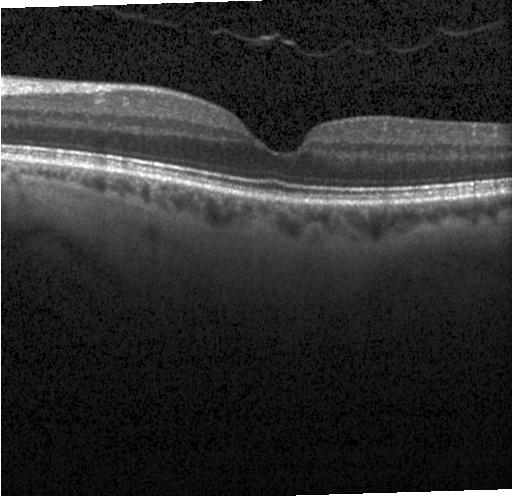

Spectral-domain optical coherence tomography · OCT B-scan · through the macula
Diagnosis: neither choroidal neovascularization, diabetic macular edema, nor drusen.